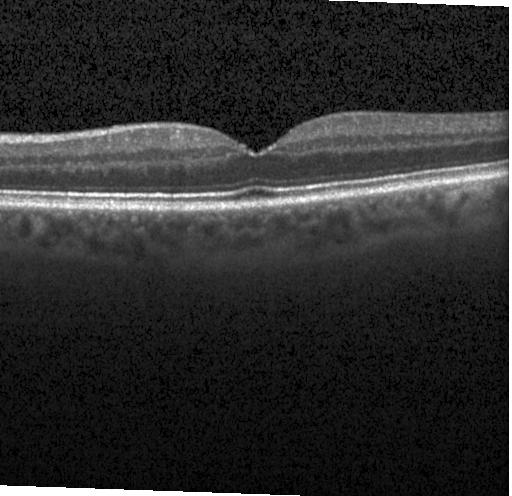
Retinal OCT B-scan · Heidelberg Spectralis OCT system · spectral-domain optical coherence tomography · macular scan — Finding: no evidence of choroidal neovascularization, diabetic macular edema, or drusen.